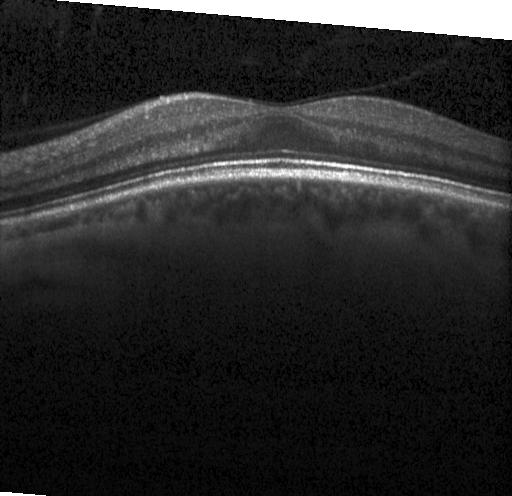

The scan shows no choroidal neovascularization, no diabetic macular edema, and no drusen.